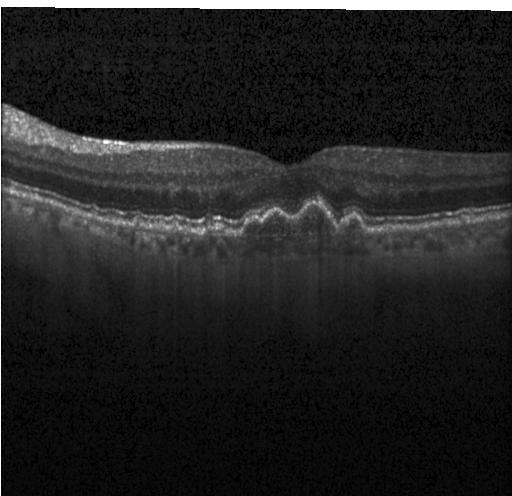 Optical coherence tomography scan; Heidelberg Spectralis OCT system — OCT finding: sub-RPE drusenoid deposits.